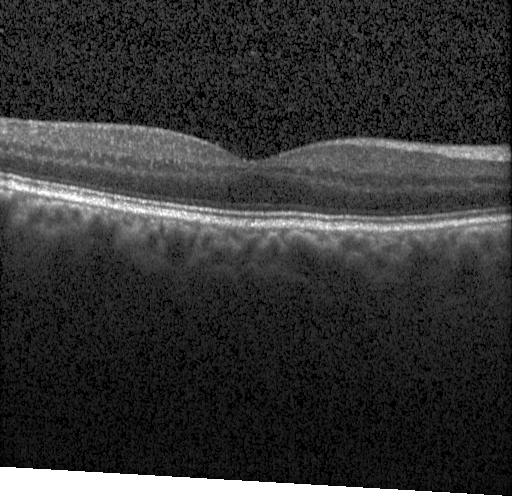 Macular OCT: no choroidal neovascularization, diabetic macular edema, or drusen.